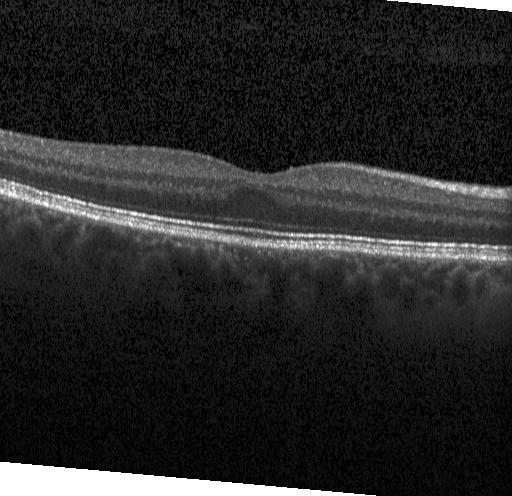

Finding: no choroidal neovascularization, no diabetic macular edema, and no drusen.